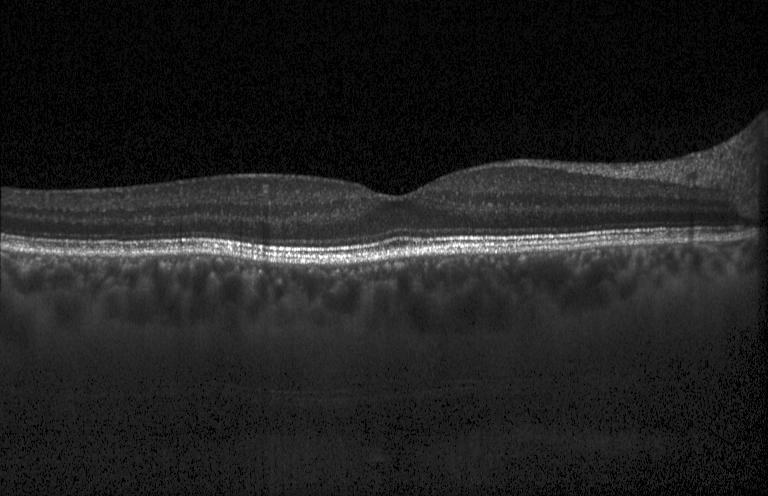
Acquired on a Heidelberg Spectralis, centered on the fovea, SD-OCT, optical coherence tomography B-scan
Finding: neither choroidal neovascularization, diabetic macular edema, nor drusen.